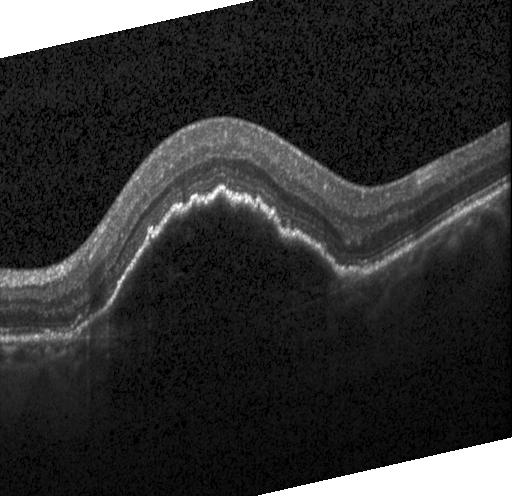

A choroidal neovascular membrane.